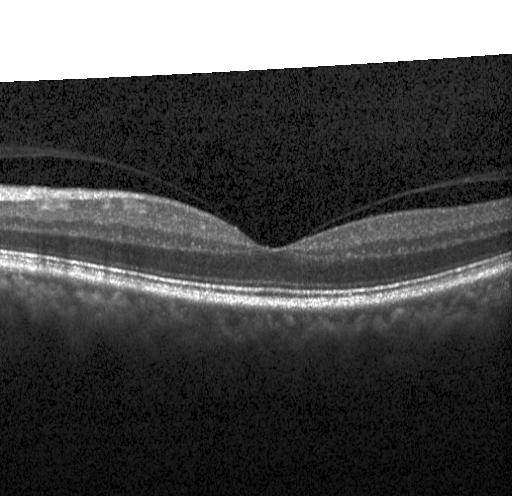
Heidelberg Spectralis; retinal OCT B-scan; SD-OCT. Finding: no choroidal neovascularization, diabetic macular edema, or drusen.